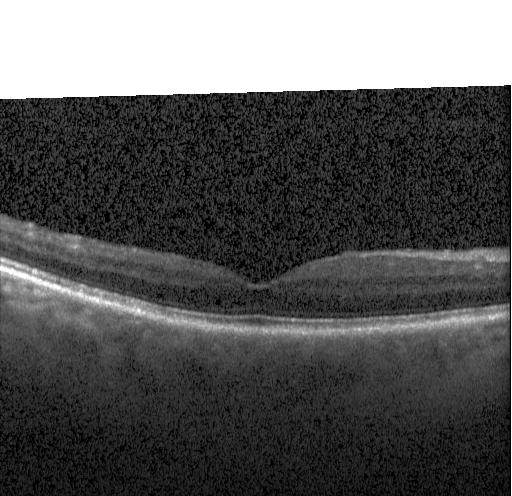

Optical coherence tomography B-scan; SD-OCT; Heidelberg Spectralis OCT system; through the macula. Impression: no evidence of choroidal neovascularization, diabetic macular edema, or drusen.